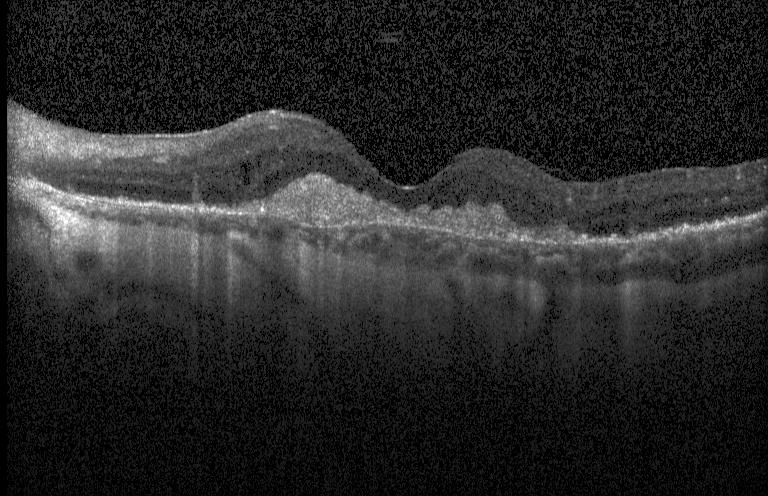

Centered on the fovea, instrument: Heidelberg Spectralis, spectral-domain OCT, optical coherence tomography scan.
Assessment: a choroidal neovascular membrane.